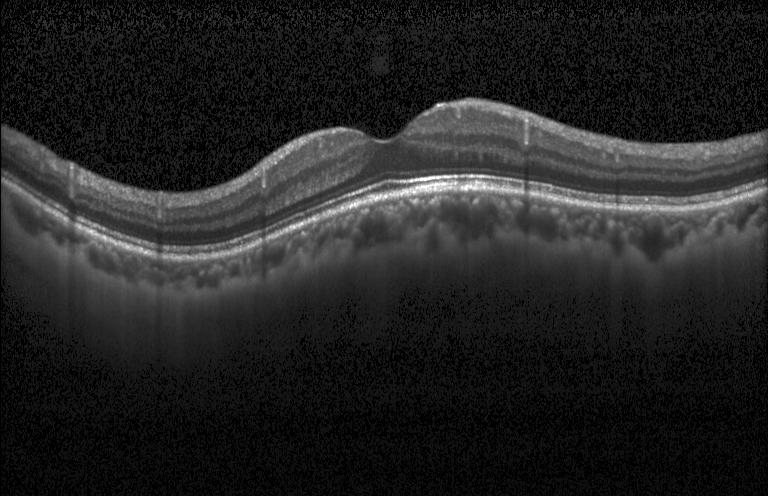 Optical coherence tomography scan · horizontal scan through the fovea. Finding: no evidence of CNV, DME, or drusen.